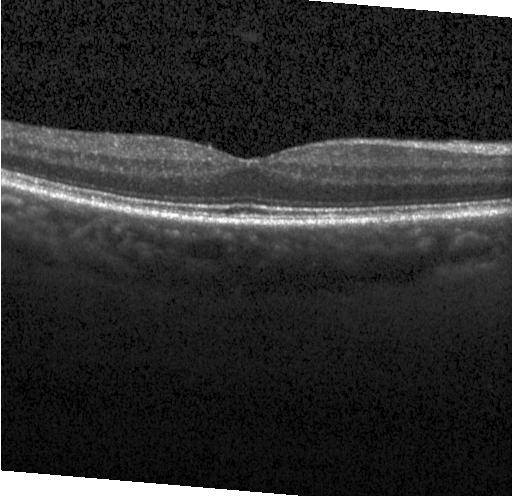 Impression: no CNV, DME, or drusen.